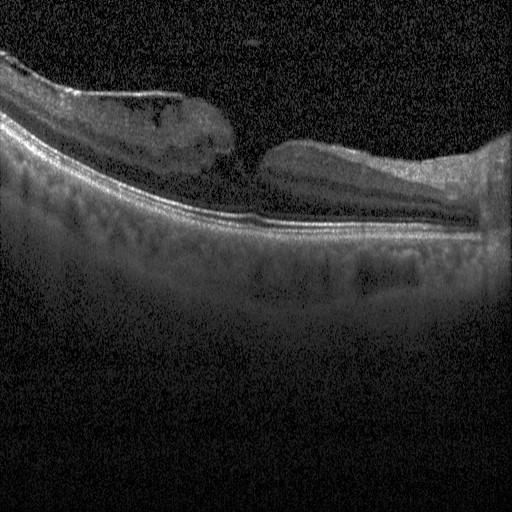

Dx: diabetic macular edema.